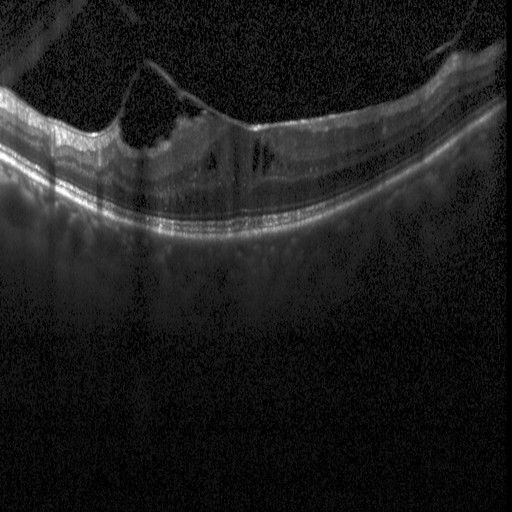

Spectral-domain optical coherence tomography. Instrument: Heidelberg Spectralis. Optical coherence tomography B-scan. Fovea-centered — This B-scan demonstrates diabetic macular edema (DME).